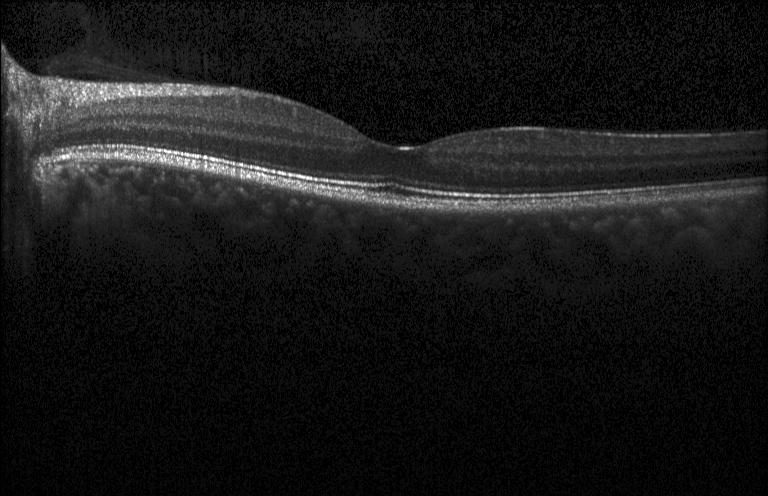
OCT B-scan, SD-OCT.
Impression: no CNV, no DME, and no drusen.